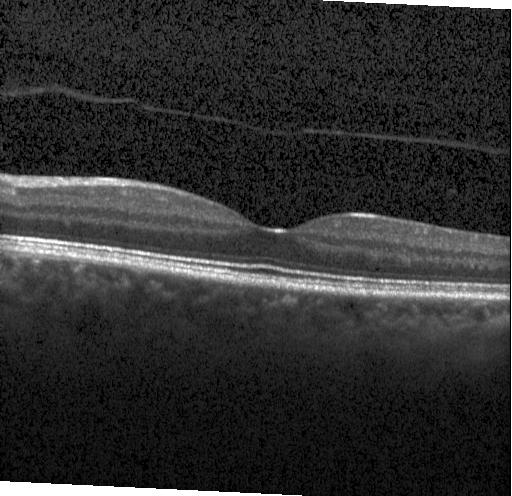 OCT B-scan, SD-OCT — No choroidal neovascularization, diabetic macular edema, or drusen.